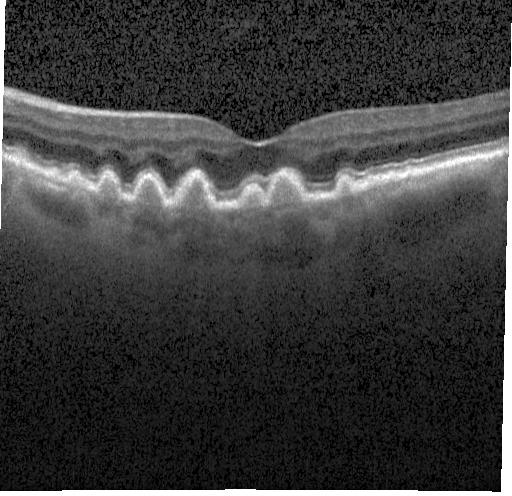

Centered on the fovea · OCT line scan · spectral-domain optical coherence tomography
Finding: sub-RPE drusenoid deposits.